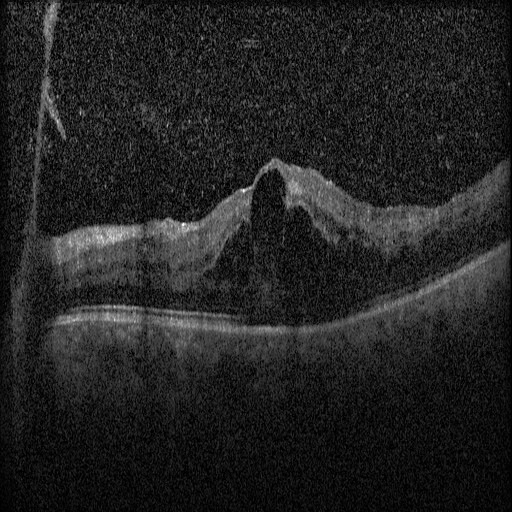 The scan shows diabetic macular edema (DME).